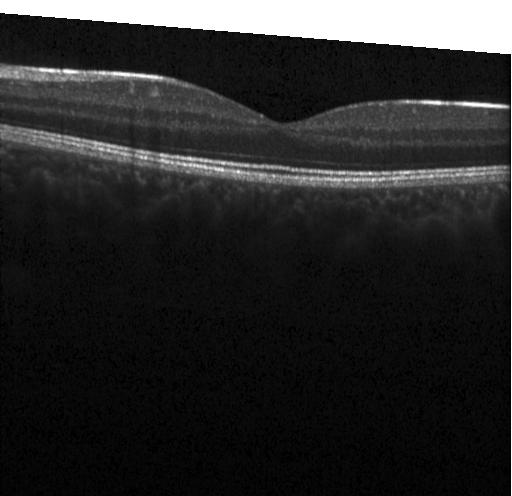
Macular OCT: no choroidal neovascularization, diabetic macular edema, or drusen.